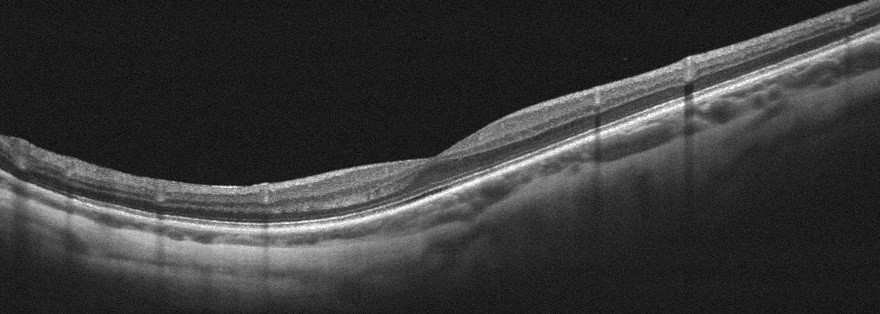

Retinal OCT B-scan. No AMD, DME, ERM, RAO, RVO, or VID.